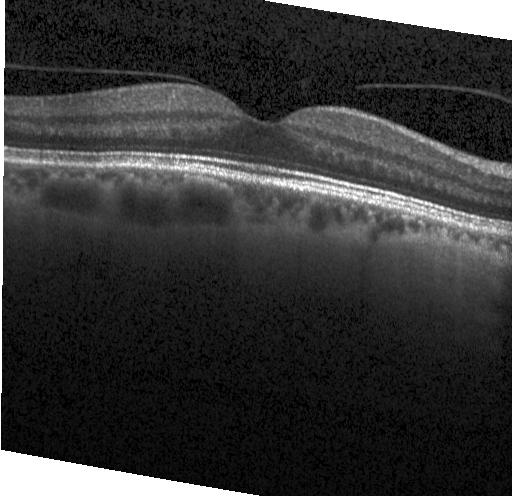
The scan shows no choroidal neovascularization, no diabetic macular edema, and no drusen.